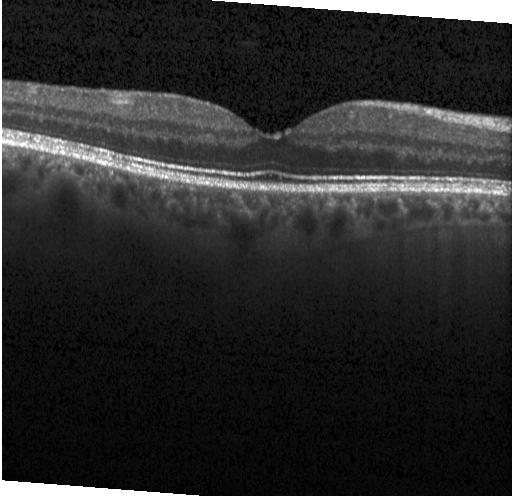 OCT B-scan showing no evidence of choroidal neovascularization, diabetic macular edema, or drusen.